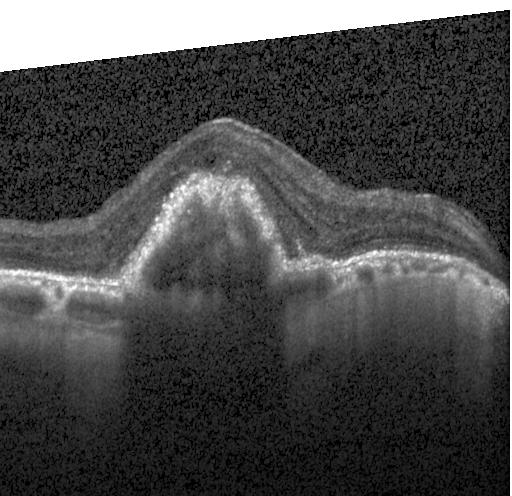

Heidelberg Spectralis · OCT B-scan · centered on the fovea · SD-OCT.
Impression: a choroidal neovascular membrane.